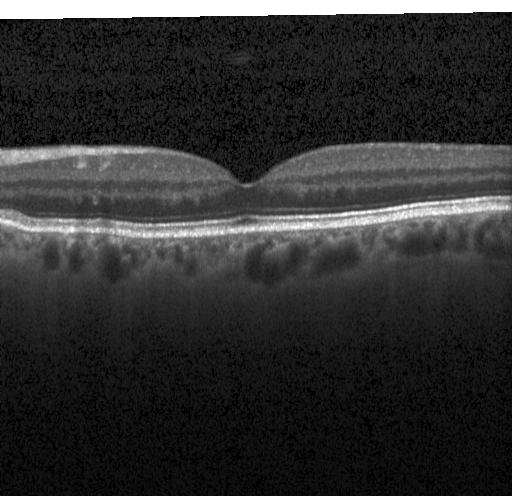
Macular OCT: no choroidal neovascularization, diabetic macular edema, or drusen.